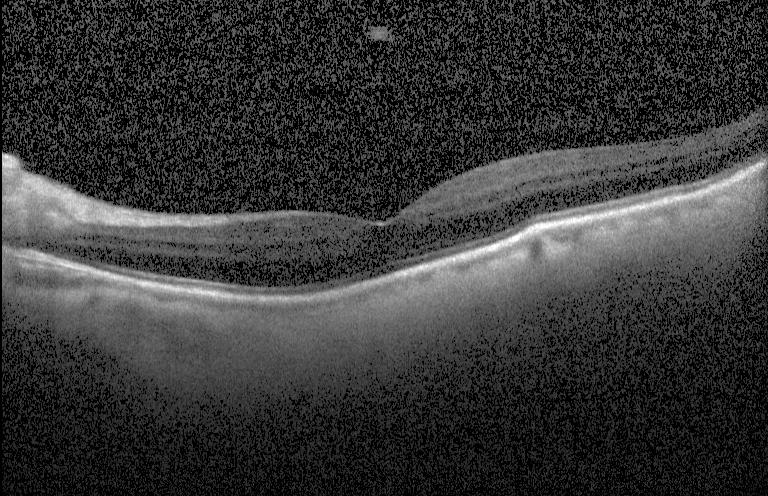 Heidelberg Spectralis; retinal OCT cross-section; centered on the fovea; spectral-domain OCT.
Finding: no choroidal neovascularization, diabetic macular edema, or drusen.